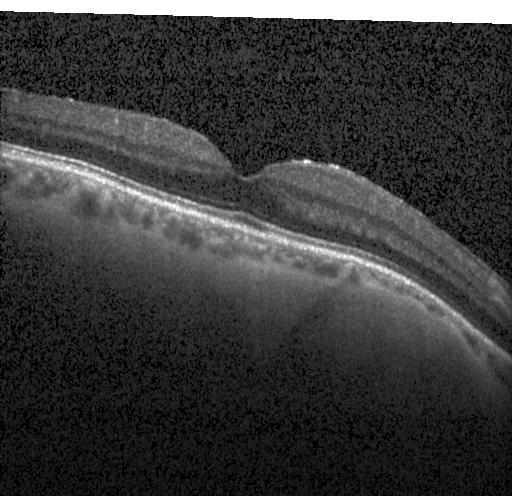

Assessment: no choroidal neovascularization, diabetic macular edema, or drusen.